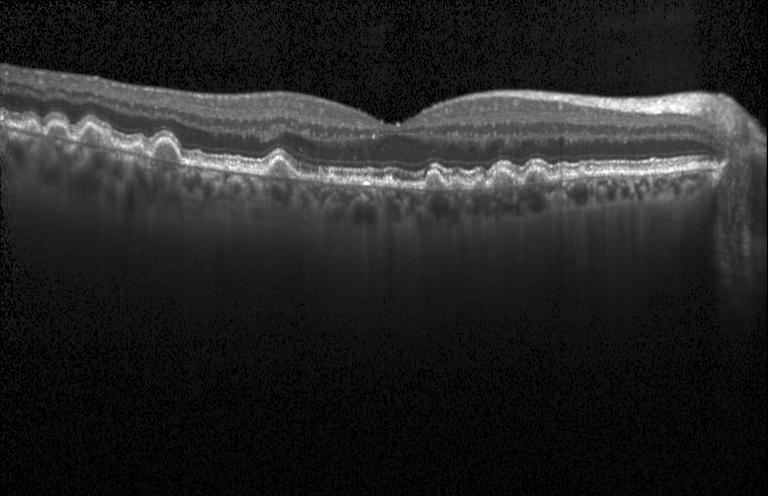
Retinal OCT B-scan; instrument: Heidelberg Spectralis; spectral-domain optical coherence tomography; horizontal scan through the fovea.
Assessment: multiple drusen.